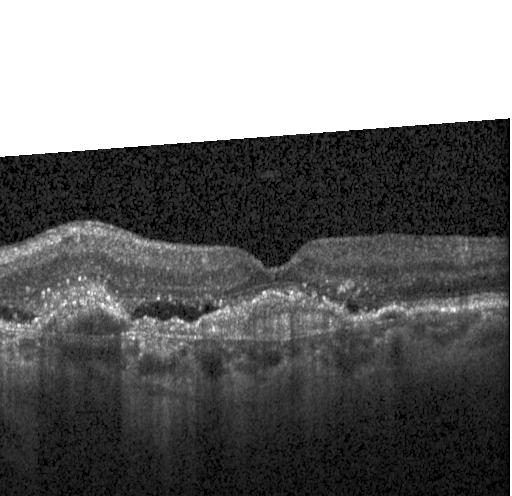

Macular OCT: choroidal neovascularization.